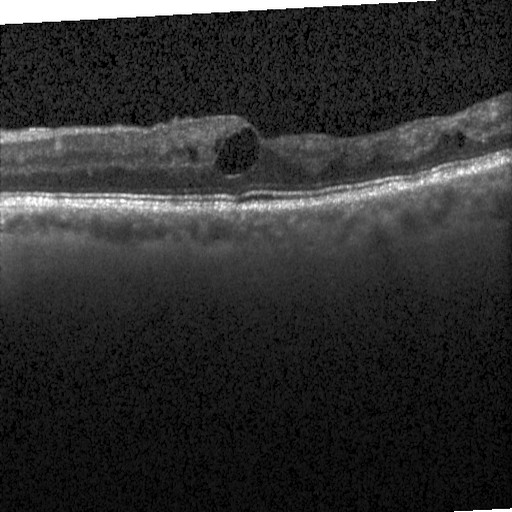

Heidelberg Spectralis · spectral-domain optical coherence tomography · OCT B-scan
Impression: DME.